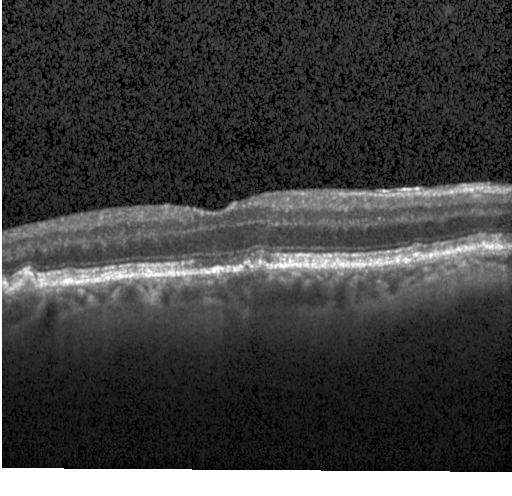

OCT scan showing drusen.